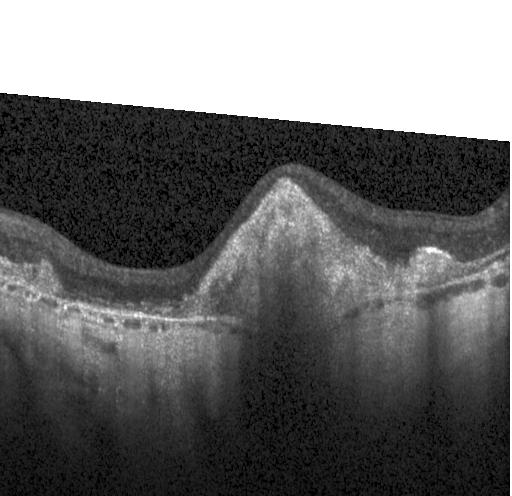

Optical coherence tomography scan — Impression: a choroidal neovascular membrane.